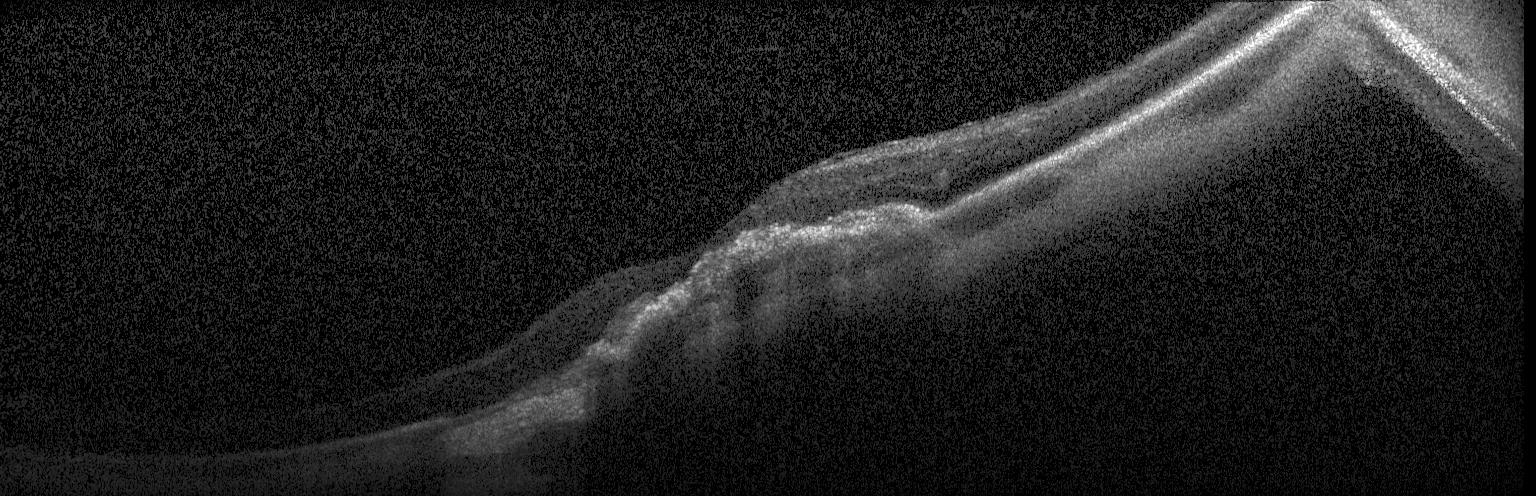 Instrument: Heidelberg Spectralis, OCT line scan, SD-OCT, horizontal scan through the fovea. Diagnosis: choroidal neovascularization.